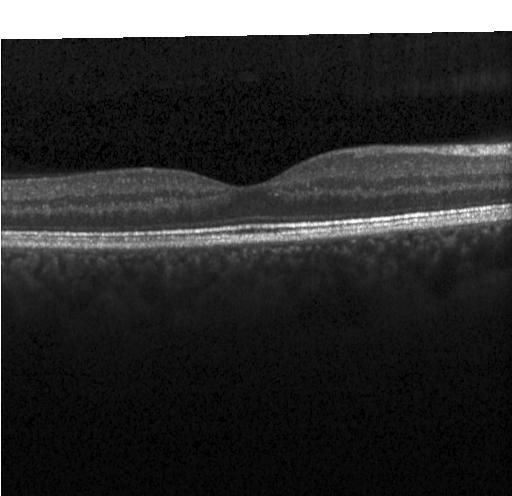 Horizontal scan through the fovea; optical coherence tomography B-scan — Neither choroidal neovascularization, diabetic macular edema, nor drusen.